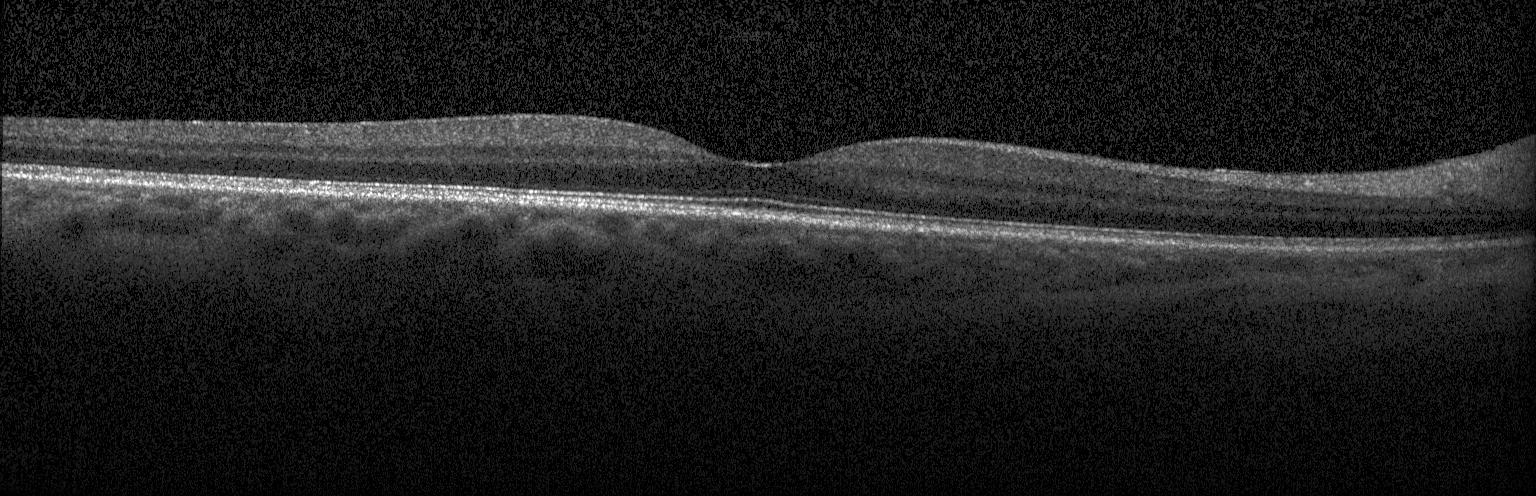

Spectral-domain OCT B-scan: no choroidal neovascularization, diabetic macular edema, or drusen.